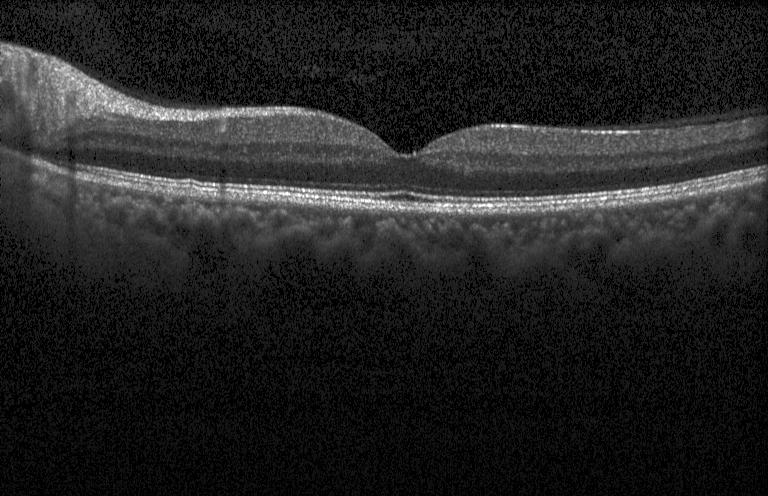 OCT line scan. The scan shows no CNV, DME, or drusen.